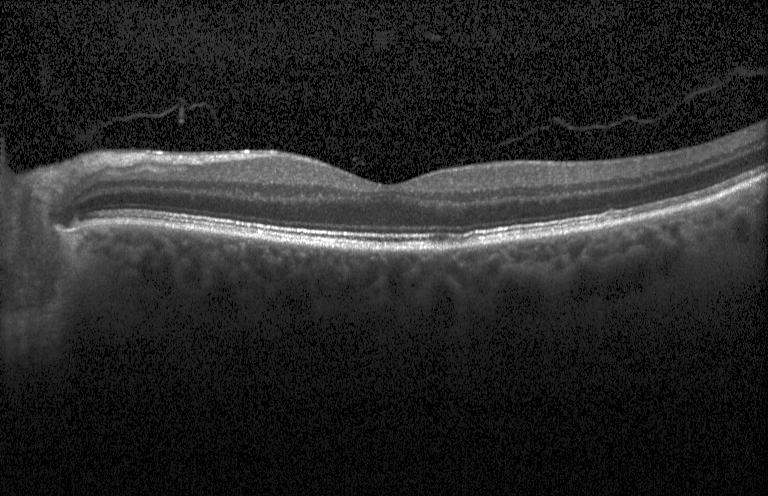 Macular scan; optical coherence tomography B-scan. Diagnosis: neither choroidal neovascularization, diabetic macular edema, nor drusen.